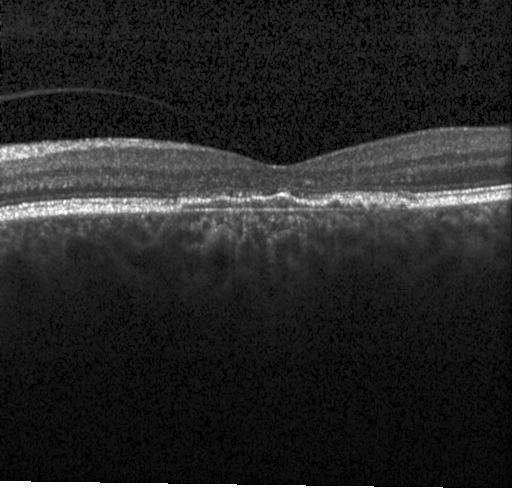

Acquired on a Heidelberg Spectralis. OCT line scan. Spectral-domain optical coherence tomography. Centered on the fovea. This B-scan demonstrates CNV.